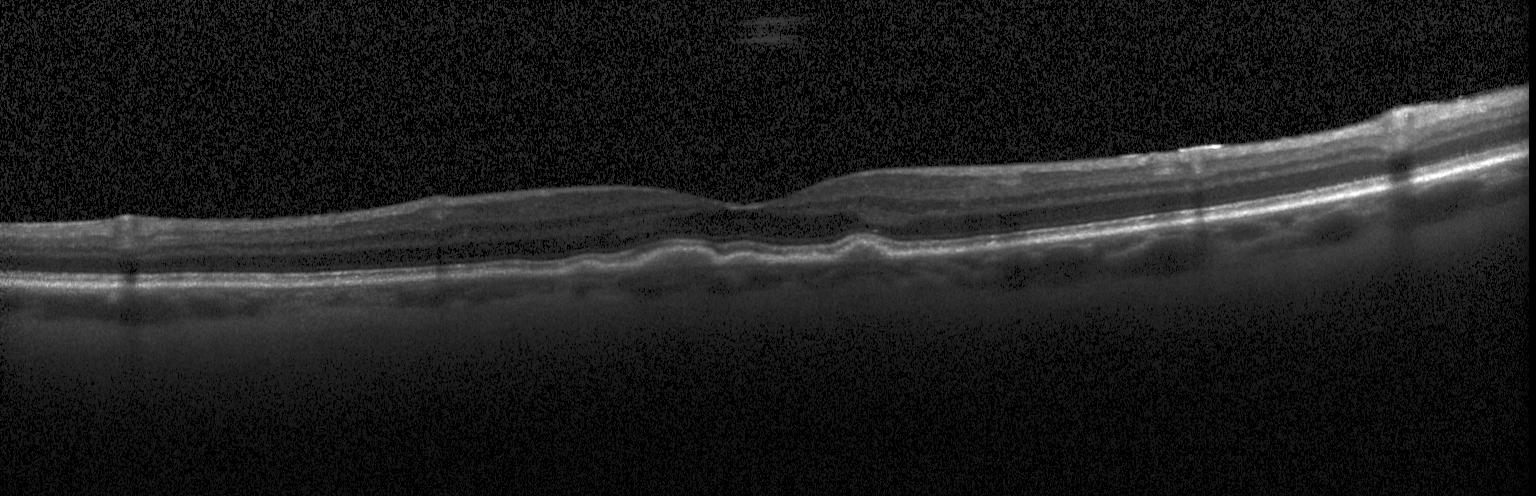 OCT finding: sub-RPE drusenoid deposits.